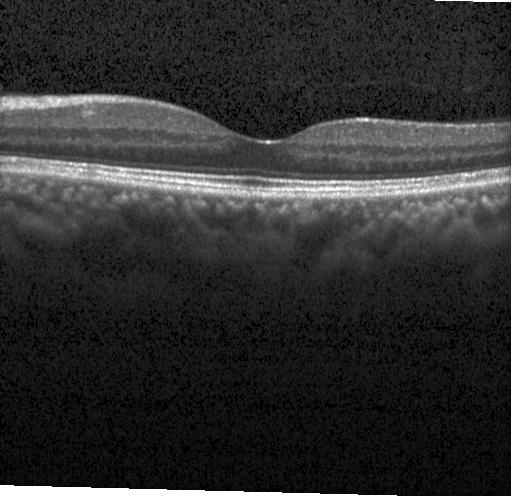 Finding: no CNV, DME, or drusen.